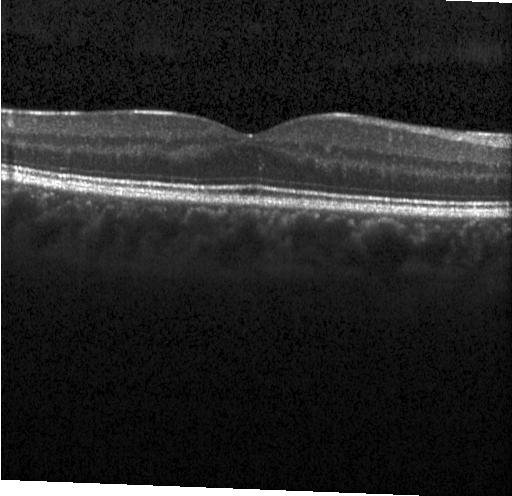
Heidelberg Spectralis OCT system. Optical coherence tomography scan. Spectral-domain OCT
The scan shows no CNV, no DME, and no drusen.